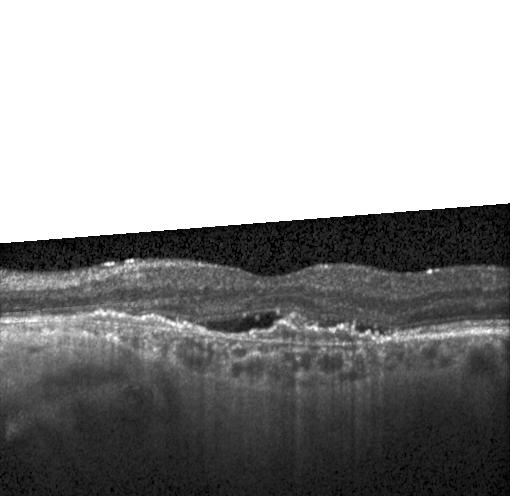 Spectral-domain optical coherence tomography; optical coherence tomography scan — A choroidal neovascular membrane.